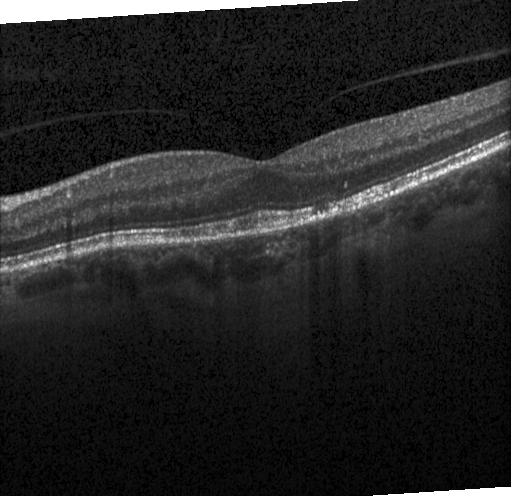
Through the macula, optical coherence tomography B-scan, Heidelberg Spectralis OCT system.
Diagnosis: neither choroidal neovascularization, diabetic macular edema, nor drusen.